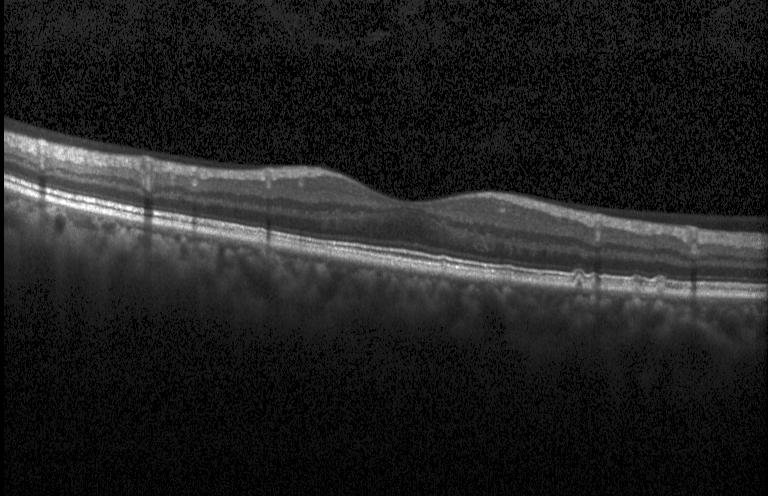

SD-OCT, retinal OCT B-scan. Sub-RPE drusenoid deposits.